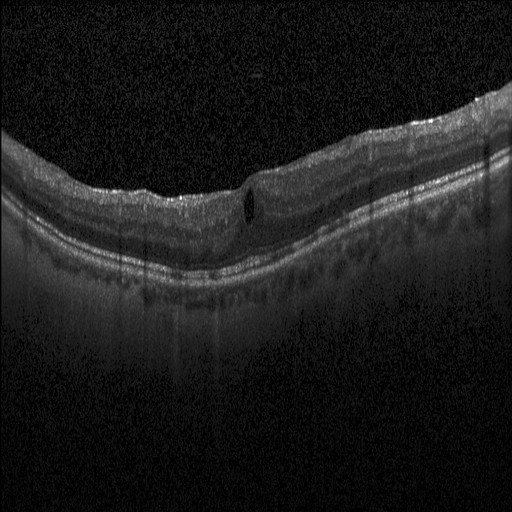
Fovea-centered, retinal OCT B-scan, Heidelberg Spectralis OCT system, spectral-domain OCT. Impression: DME.